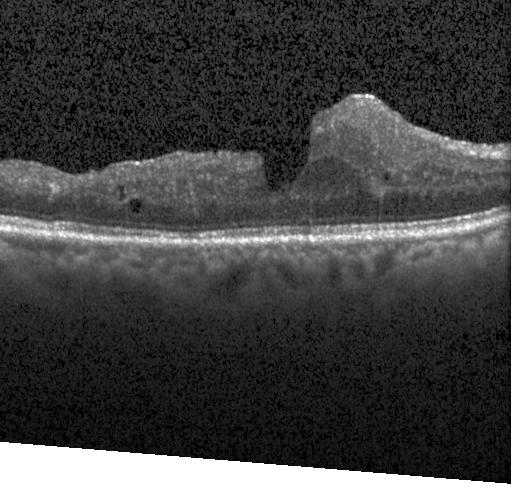
OCT scan showing diabetic macular edema (DME).